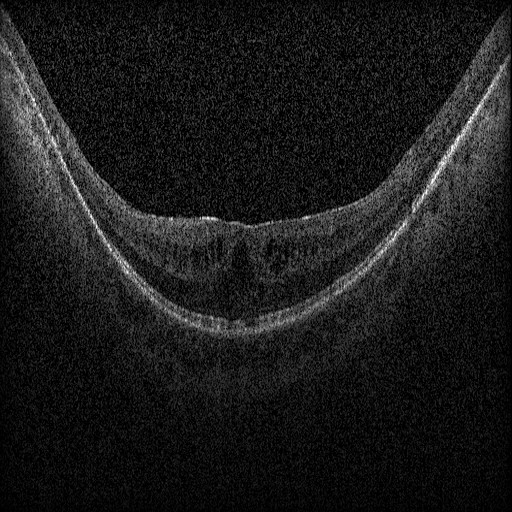
Retinal OCT cross-section — The scan shows DME.